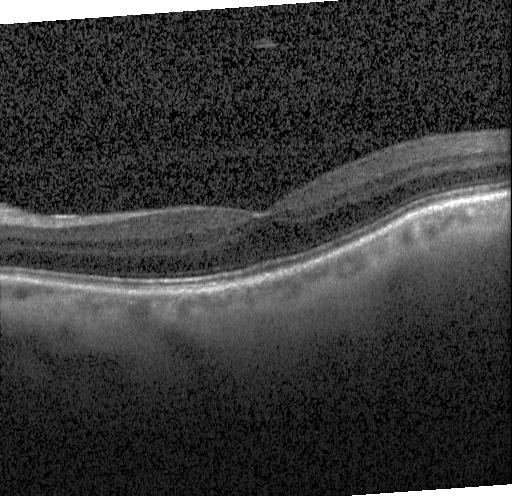

Optical coherence tomography scan. Heidelberg Spectralis OCT system. Through the macula. Spectral-domain OCT.
OCT finding: no choroidal neovascularization, no diabetic macular edema, and no drusen.